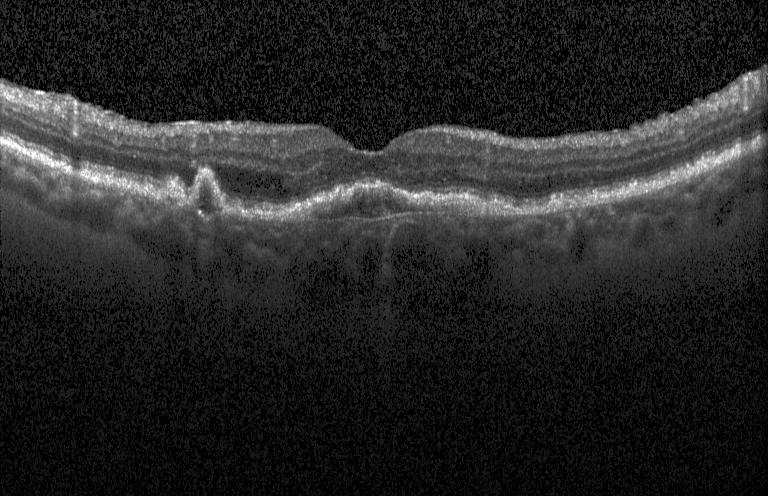
OCT B-scan showing a choroidal neovascular membrane.